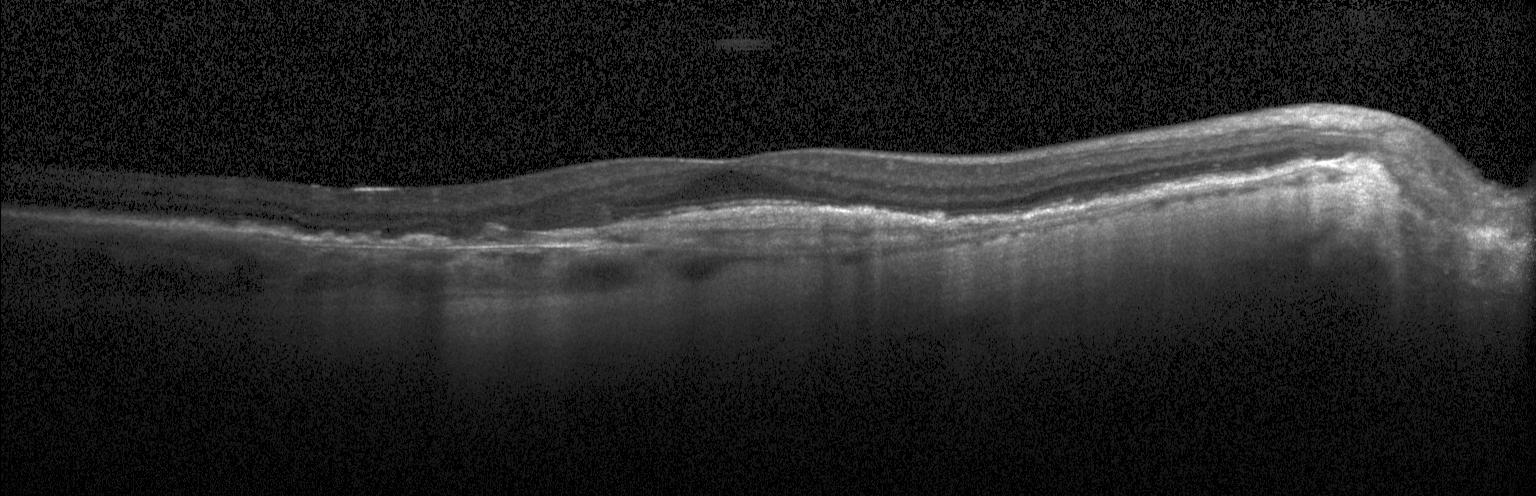 Fovea-centered; OCT B-scan; spectral-domain OCT
Diagnosis: choroidal neovascularization (CNV).